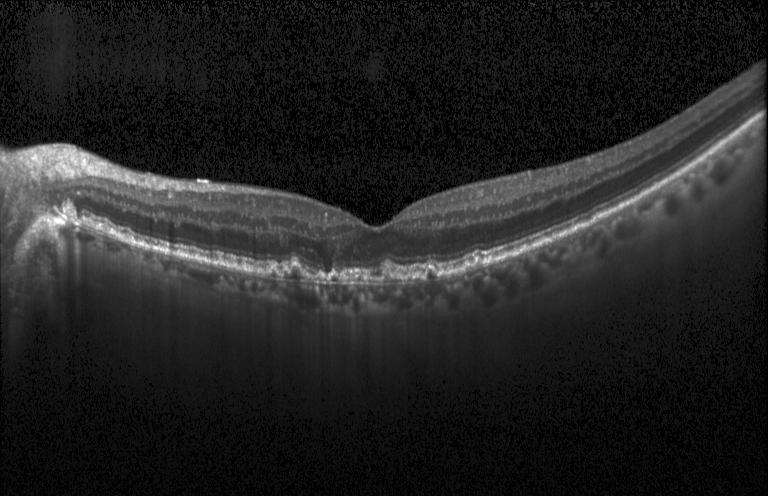 Optical coherence tomography scan · centered on the fovea · instrument: Heidelberg Spectralis · SD-OCT — Impression: drusen.